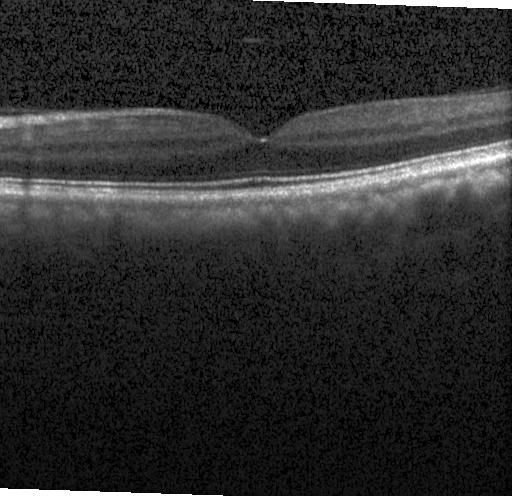 OCT B-scan; macular scan; instrument: Heidelberg Spectralis. Impression: no choroidal neovascularization, no diabetic macular edema, and no drusen.